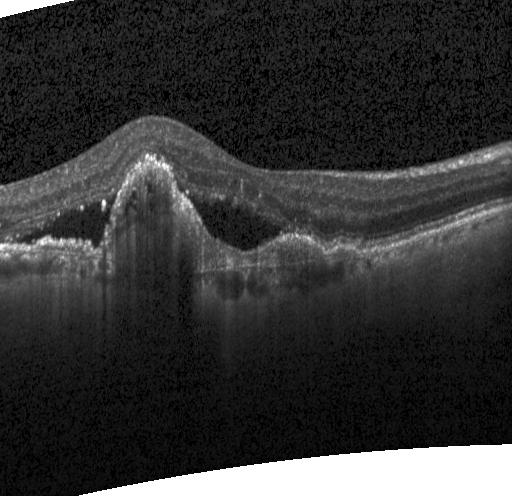 Retinal OCT cross-section — Assessment: a choroidal neovascular membrane.